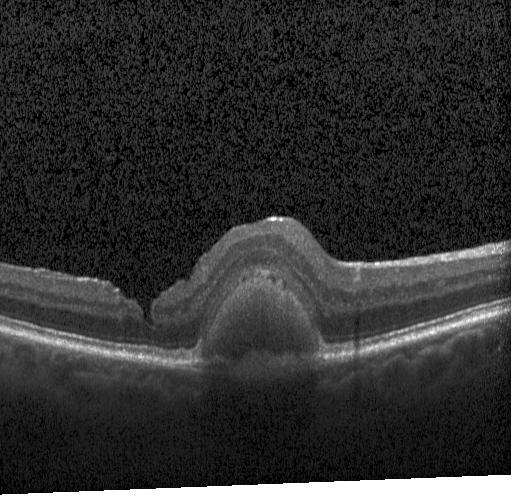 Optical coherence tomography scan.
Impression: a choroidal neovascular membrane.